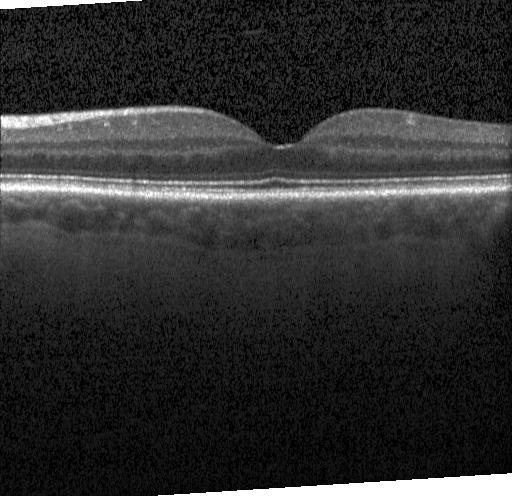
Spectral-domain OCT; centered on the fovea; optical coherence tomography B-scan; instrument: Heidelberg Spectralis — Finding: no evidence of choroidal neovascularization, diabetic macular edema, or drusen.